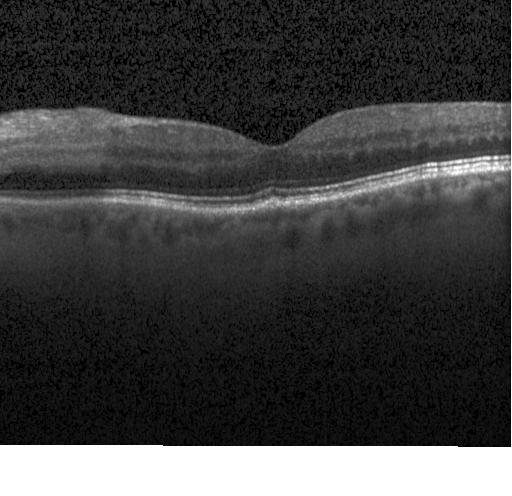 Retinal OCT cross-section. Impression: neither choroidal neovascularization, diabetic macular edema, nor drusen.